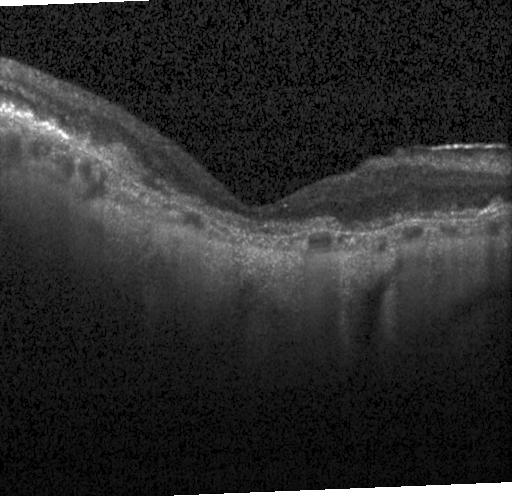

OCT line scan. Acquired on a Heidelberg Spectralis.
Assessment: a choroidal neovascular membrane.